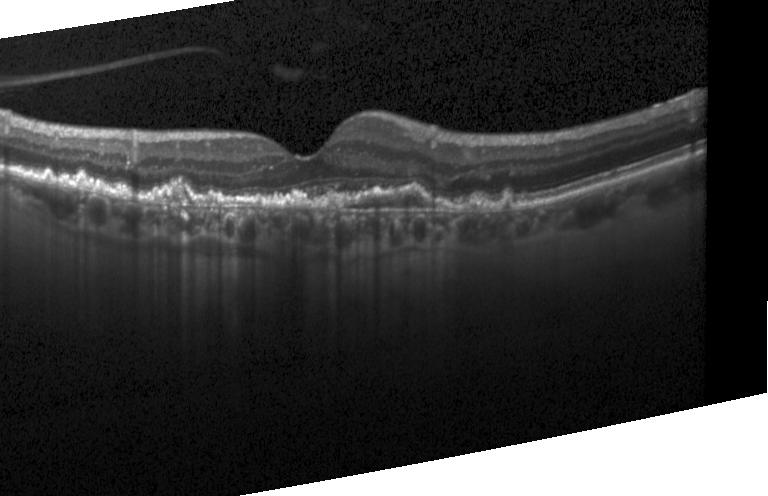
Optical coherence tomography scan — Impression: CNV.